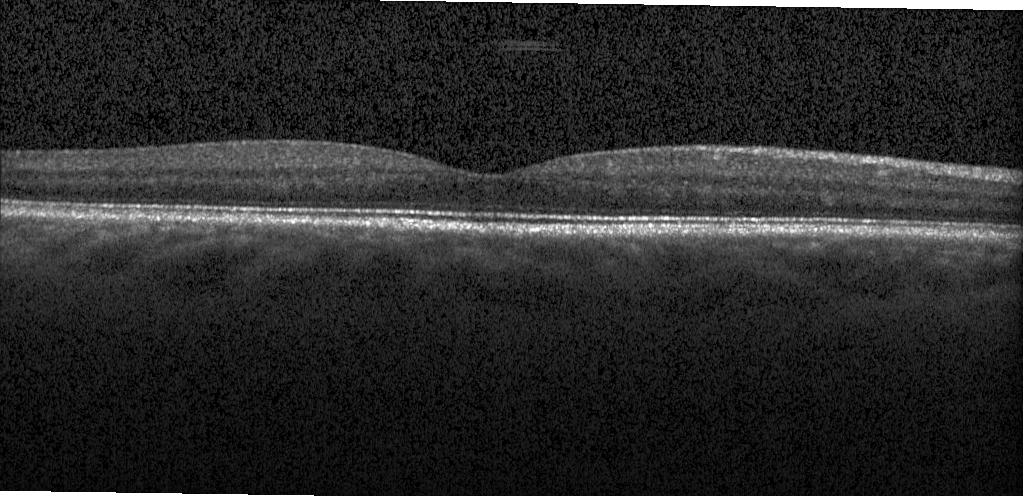 No choroidal neovascularization, diabetic macular edema, or drusen.